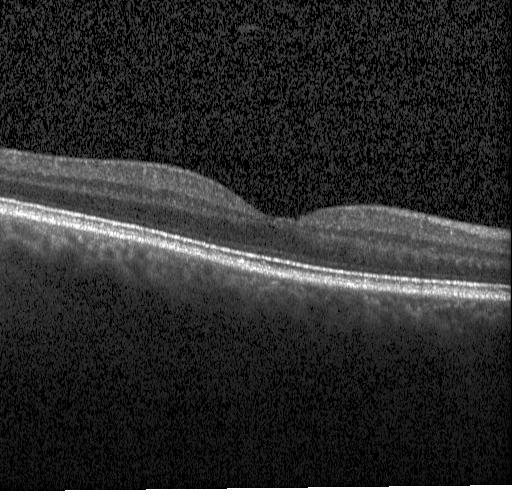 Spectral-domain optical coherence tomography. Acquired on a Heidelberg Spectralis. OCT line scan — No choroidal neovascularization, no diabetic macular edema, and no drusen.